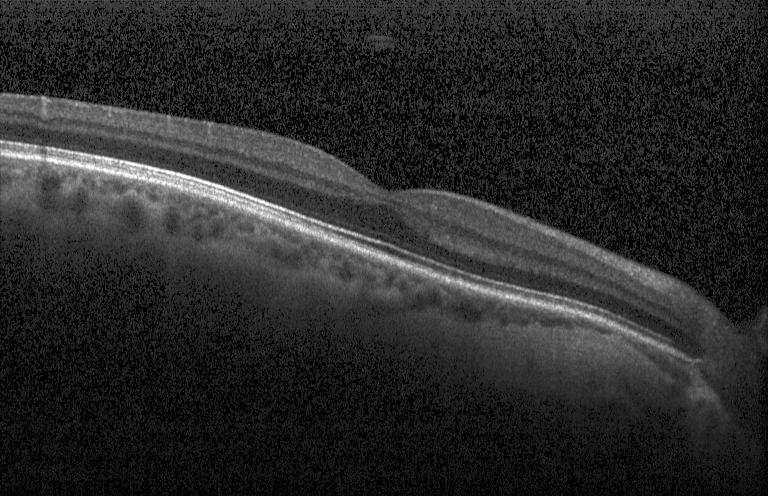 OCT line scan
OCT finding: no evidence of choroidal neovascularization, diabetic macular edema, or drusen.